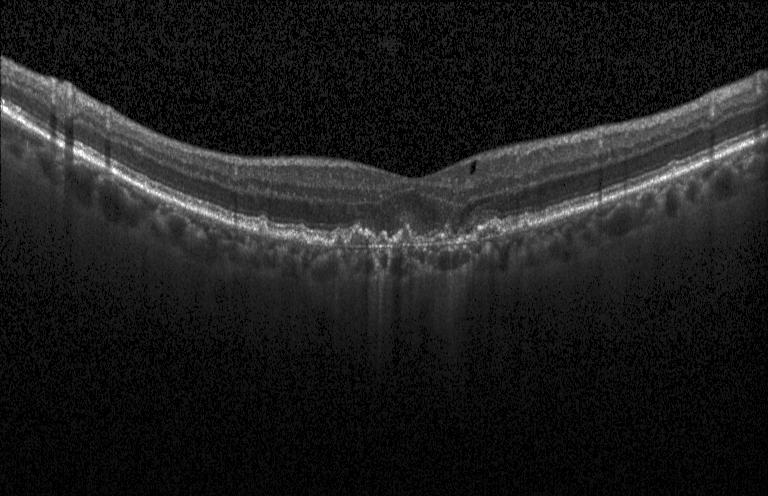

A choroidal neovascular membrane.